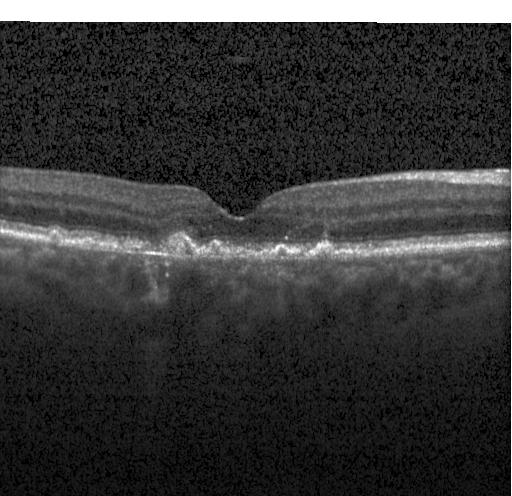

Horizontal scan through the fovea; Heidelberg Spectralis OCT system; OCT line scan; spectral-domain OCT. Diagnosis: a choroidal neovascular membrane.